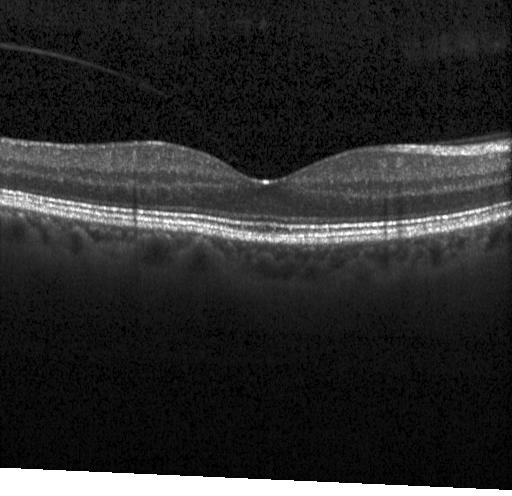
Retinal OCT cross-section.
Impression: no choroidal neovascularization, diabetic macular edema, or drusen.